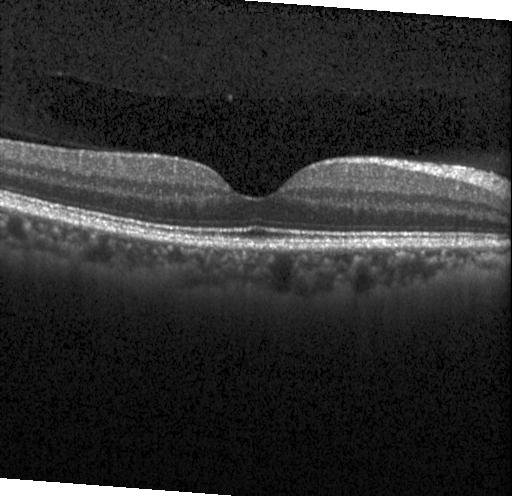
Retinal OCT cross-section showing no CNV, DME, or drusen.